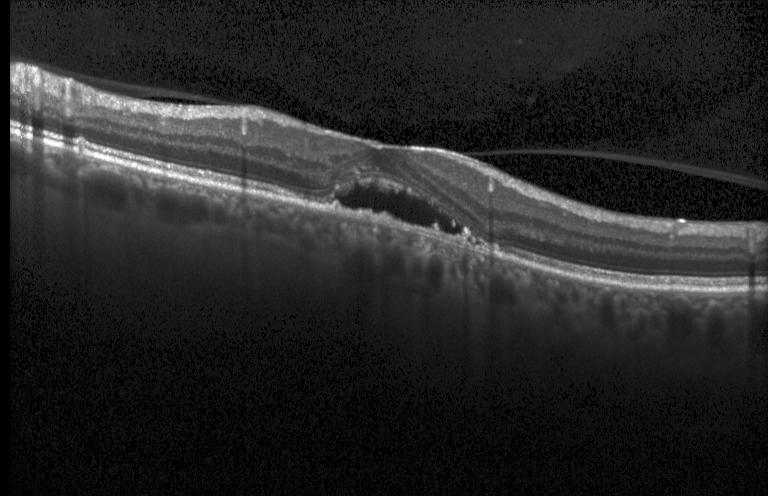

Spectral-domain OCT. Centered on the fovea. Heidelberg Spectralis. Retinal OCT cross-section. Impression: a choroidal neovascular membrane.